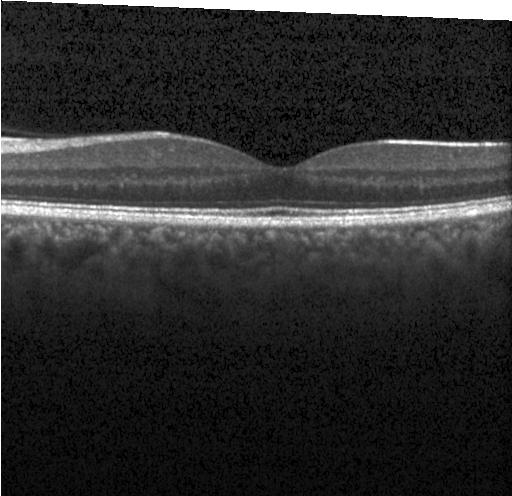

No evidence of choroidal neovascularization, diabetic macular edema, or drusen.